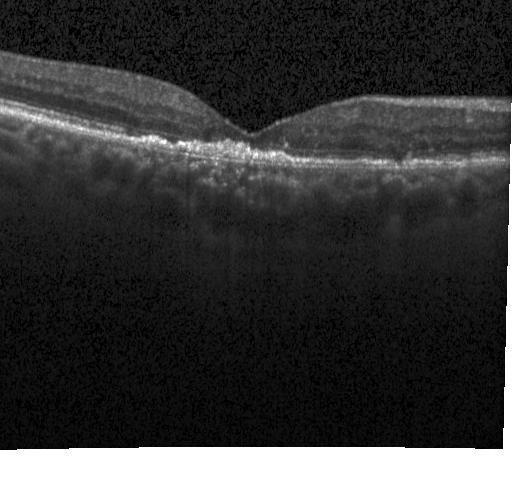

SD-OCT, through the macula, Heidelberg Spectralis OCT system, retinal OCT B-scan.
Finding: choroidal neovascularization.